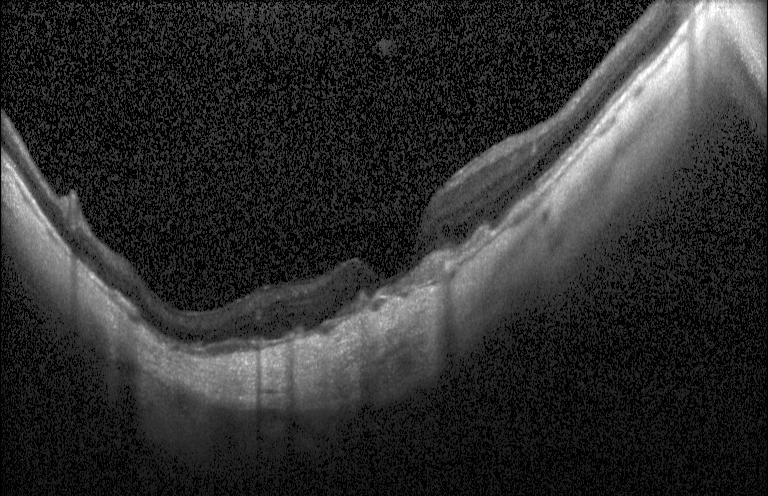 Optical coherence tomography B-scan.
OCT finding: CNV.